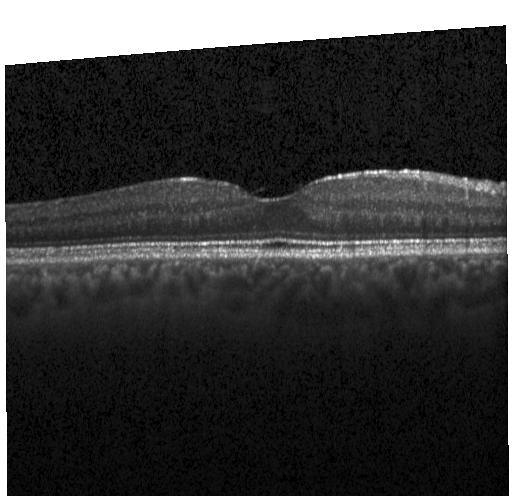 OCT scan showing no choroidal neovascularization, no diabetic macular edema, and no drusen.